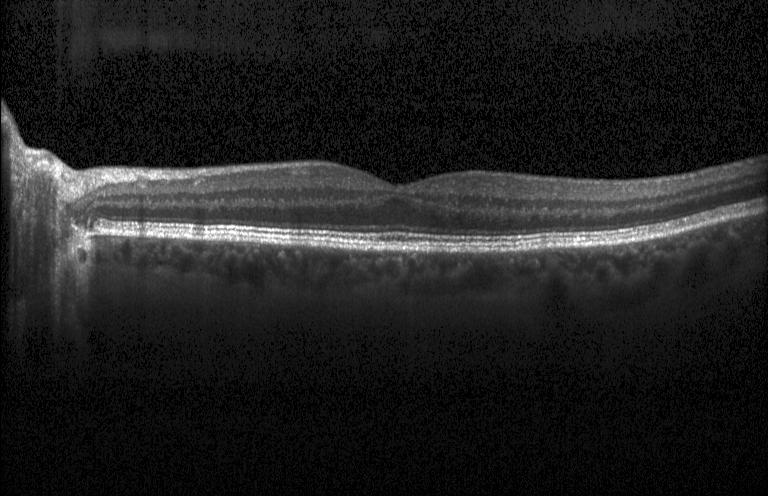

OCT finding: no choroidal neovascularization, no diabetic macular edema, and no drusen.